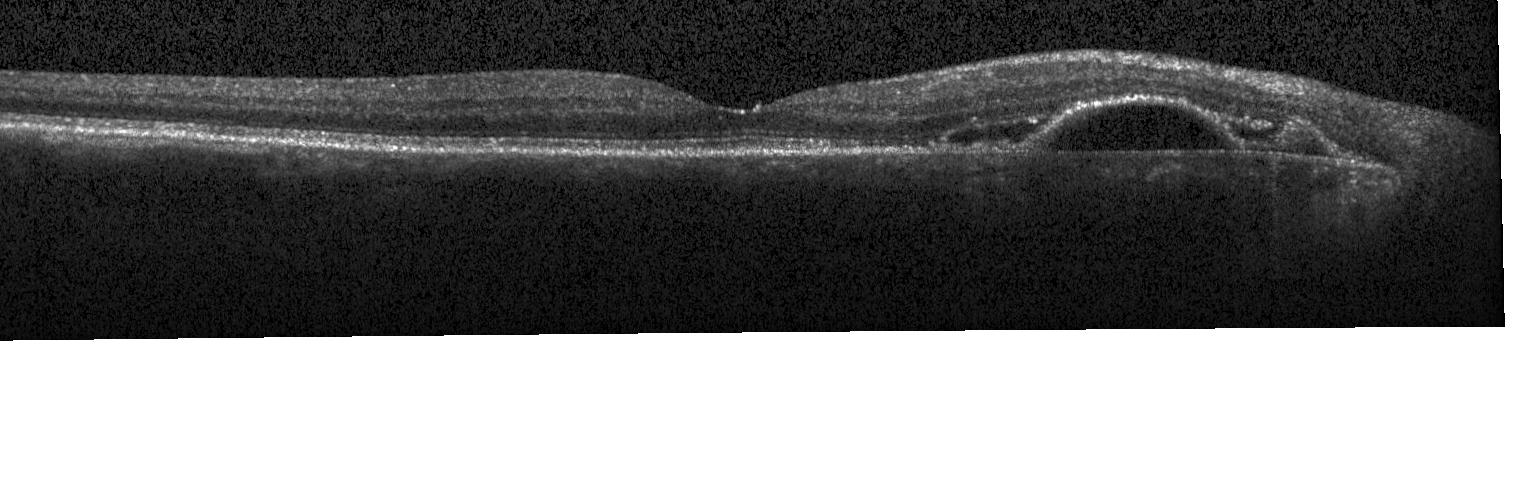
This B-scan demonstrates a choroidal neovascular membrane.